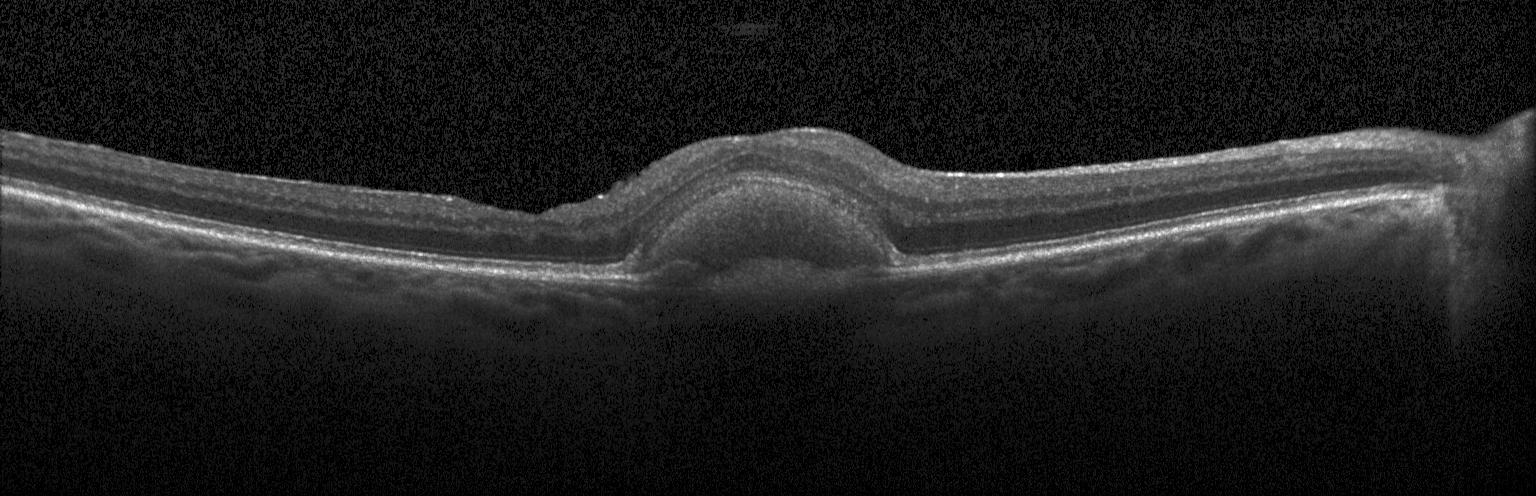

Fovea-centered · optical coherence tomography B-scan · instrument: Heidelberg Spectralis.
OCT finding: choroidal neovascularization.